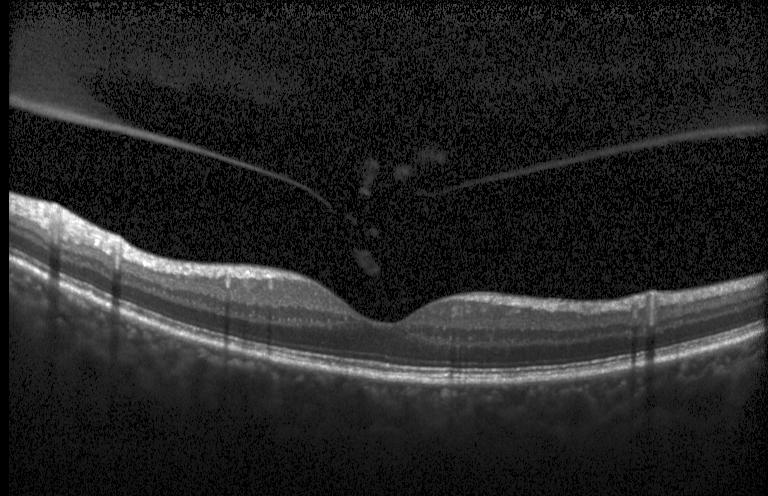

Optical coherence tomography scan. Finding: no evidence of choroidal neovascularization, diabetic macular edema, or drusen.